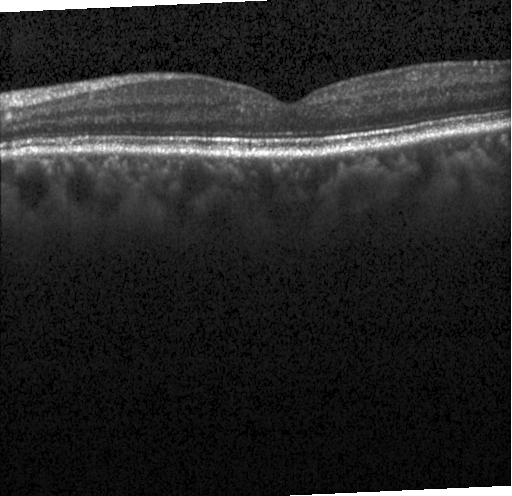

Horizontal scan through the fovea, optical coherence tomography scan — Diagnosis: no choroidal neovascularization, no diabetic macular edema, and no drusen.